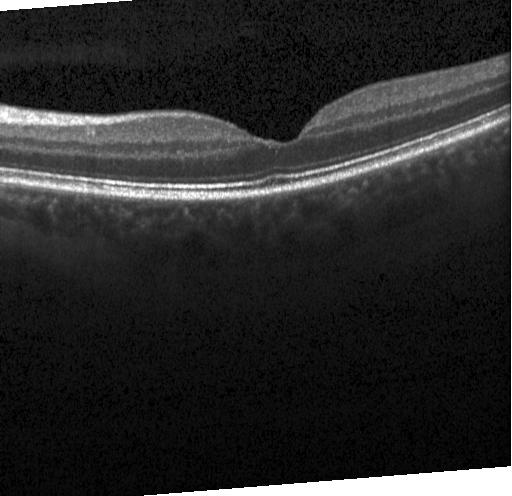

Optical coherence tomography scan; Heidelberg Spectralis; SD-OCT; fovea-centered. Impression: no evidence of CNV, DME, or drusen.